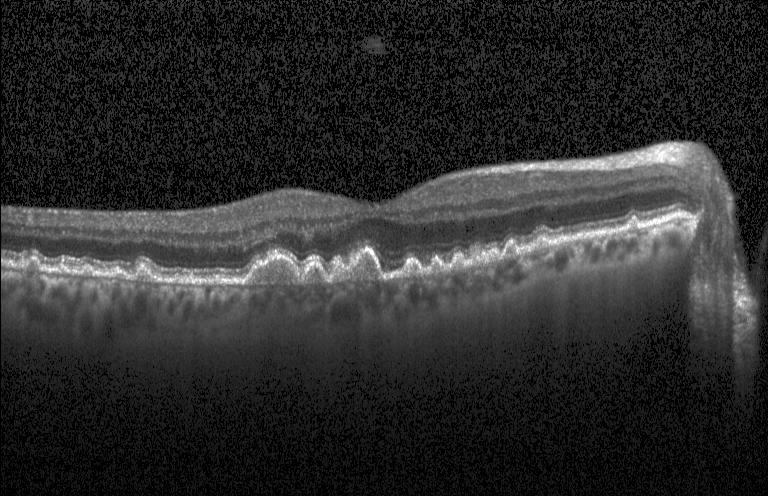 Fovea-centered, instrument: Heidelberg Spectralis, OCT B-scan
The scan shows drusen.